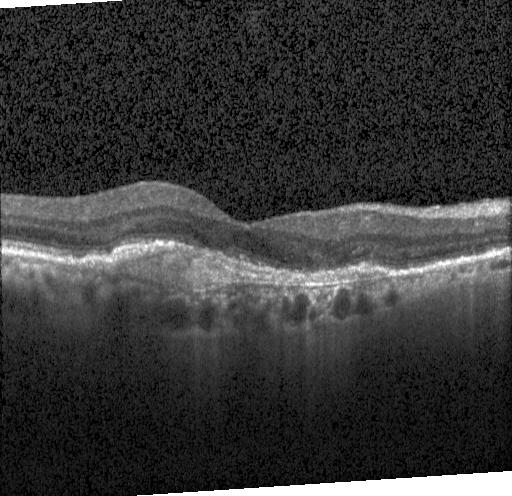 Instrument: Heidelberg Spectralis, retinal OCT B-scan
Impression: CNV.